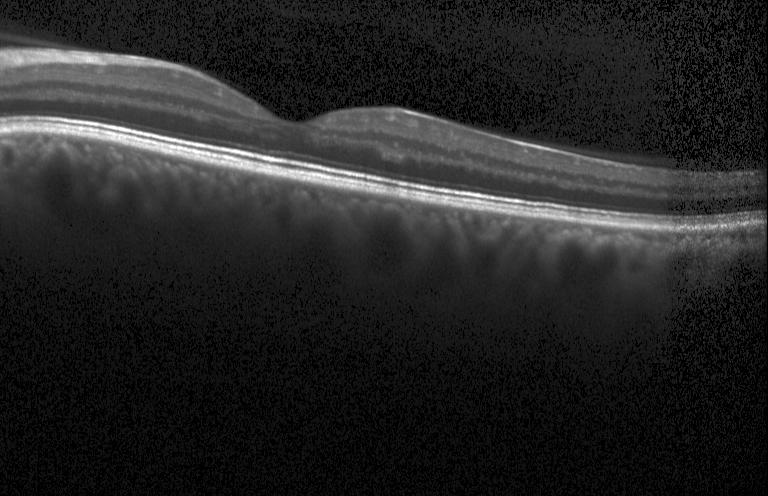
OCT scan showing no CNV, no DME, and no drusen.